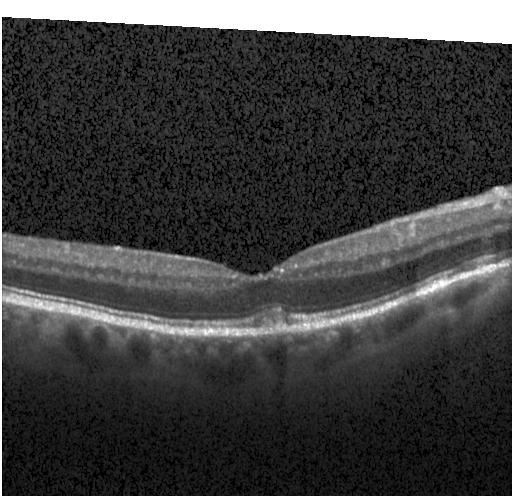

Macular OCT demonstrating drusen.